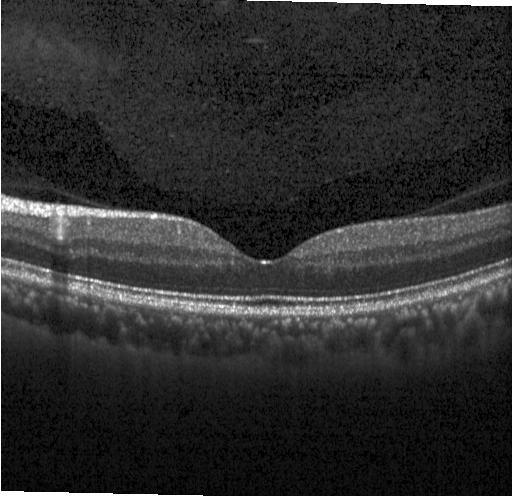
OCT B-scan; Heidelberg Spectralis OCT system; spectral-domain optical coherence tomography; centered on the fovea.
Macular OCT: no choroidal neovascularization, diabetic macular edema, or drusen.